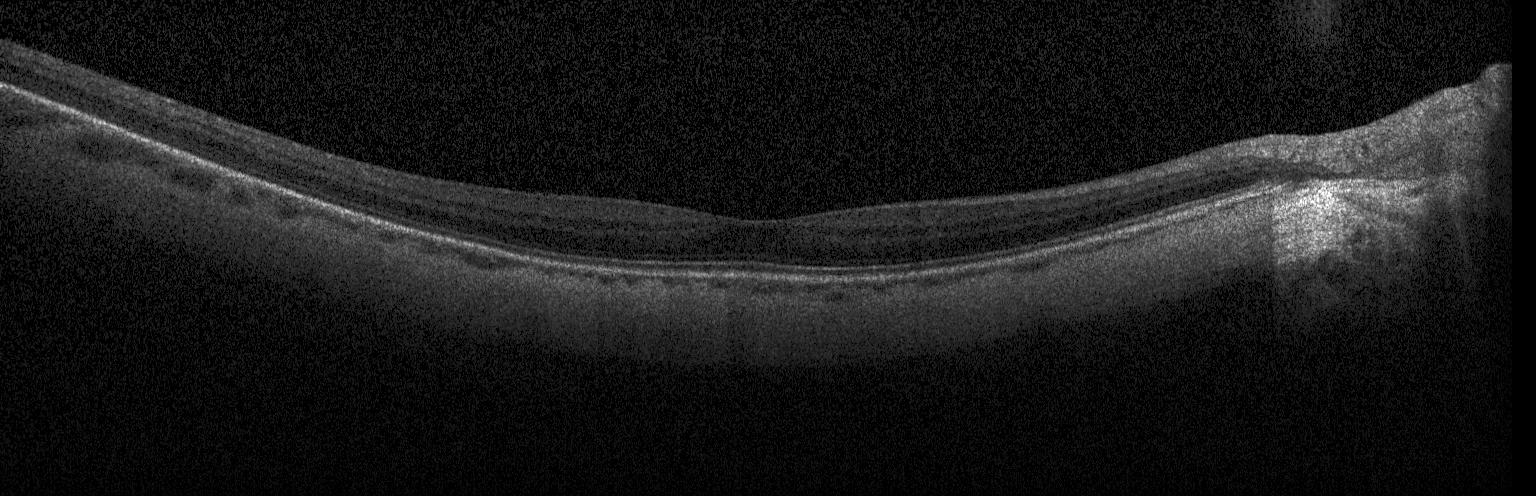 Retinal OCT cross-section
Dx: neither choroidal neovascularization, diabetic macular edema, nor drusen.